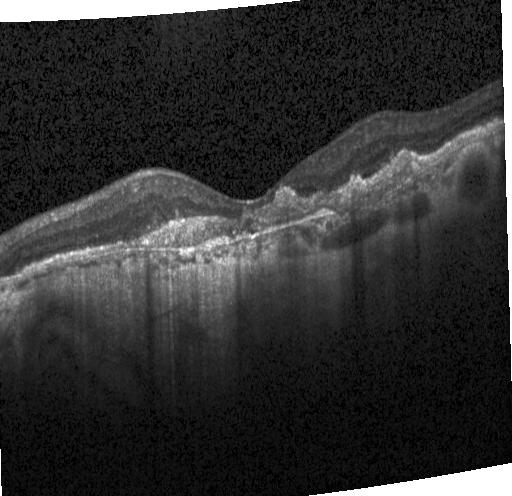 The scan shows a choroidal neovascular membrane.